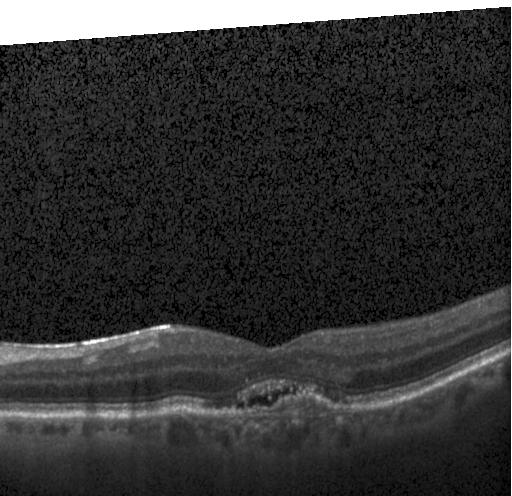
This B-scan demonstrates a choroidal neovascular membrane.